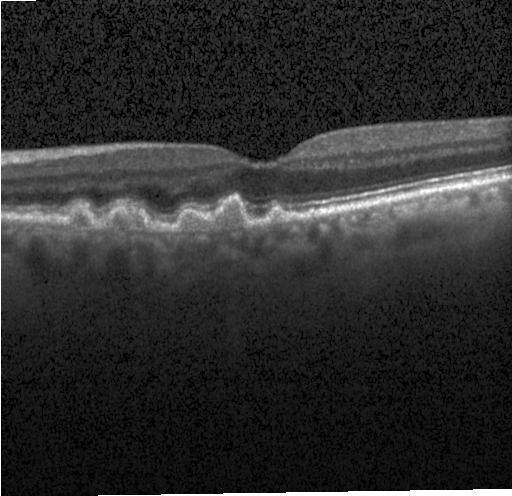 Macular scan; optical coherence tomography scan.
Sub-RPE drusenoid deposits.